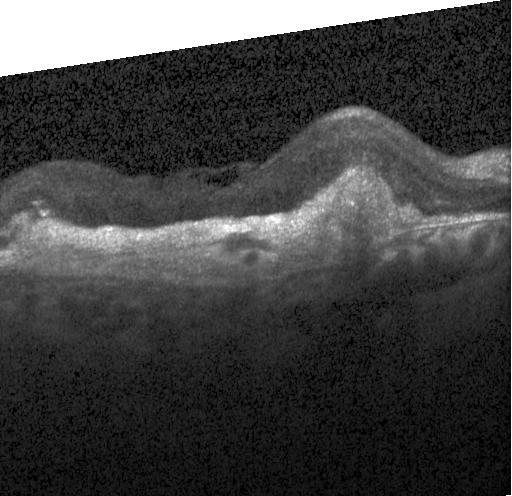
Retinal OCT B-scan. This B-scan demonstrates CNV.